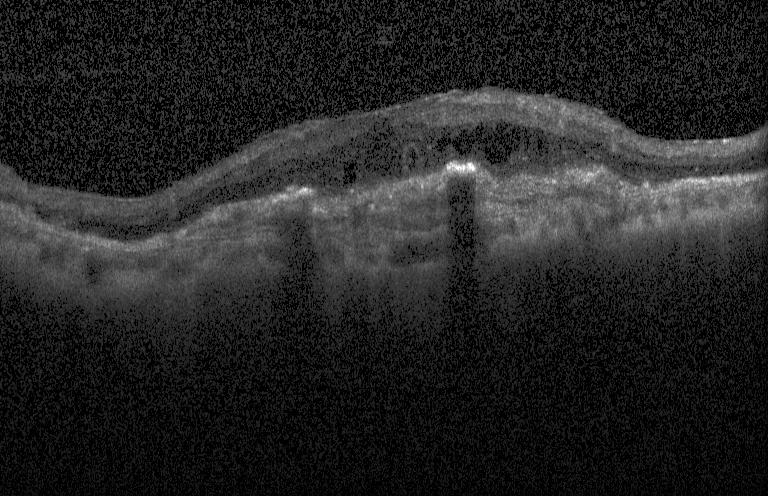 OCT line scan. SD-OCT. Instrument: Heidelberg Spectralis. Centered on the fovea — Impression: choroidal neovascularization (CNV).